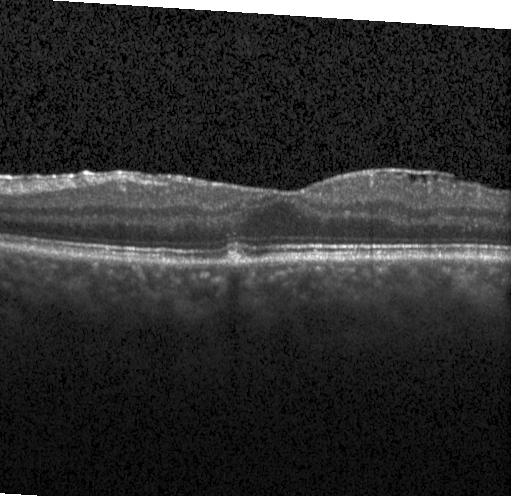 OCT B-scan, spectral-domain optical coherence tomography, acquired on a Heidelberg Spectralis, macular scan — Diagnosis: multiple drusen.